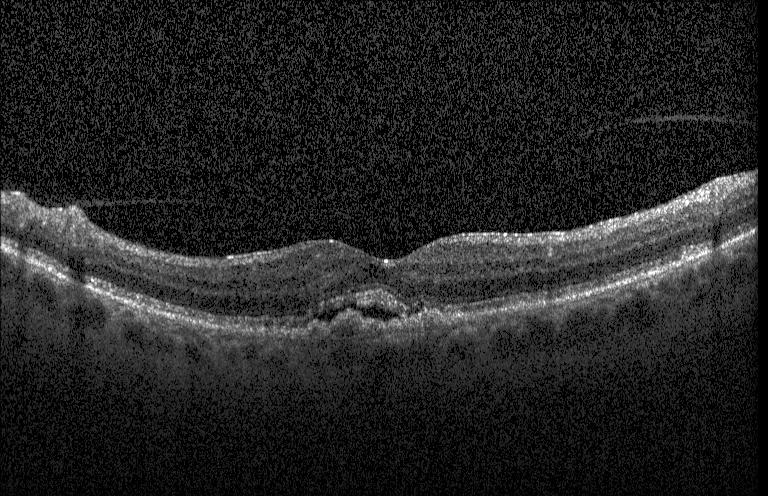
The scan shows a choroidal neovascular membrane.